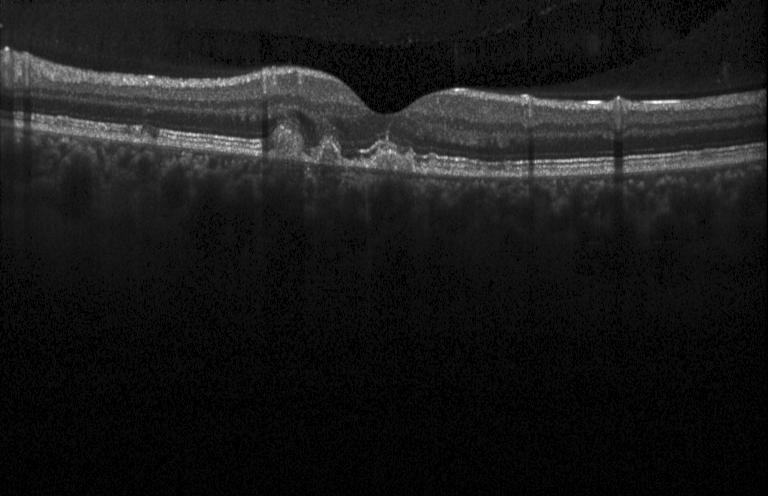

Optical coherence tomography scan, through the macula — Macular OCT: drusen.